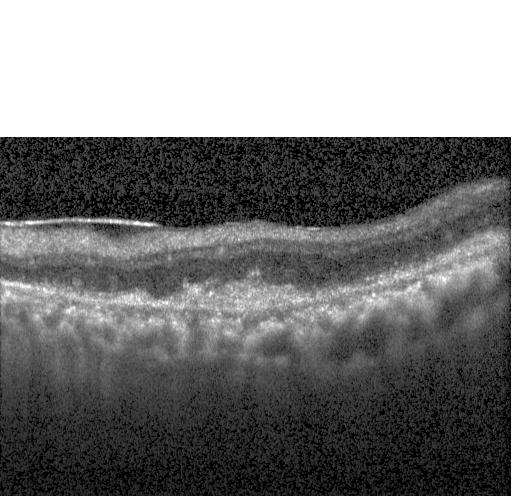 OCT B-scan showing choroidal neovascularization.